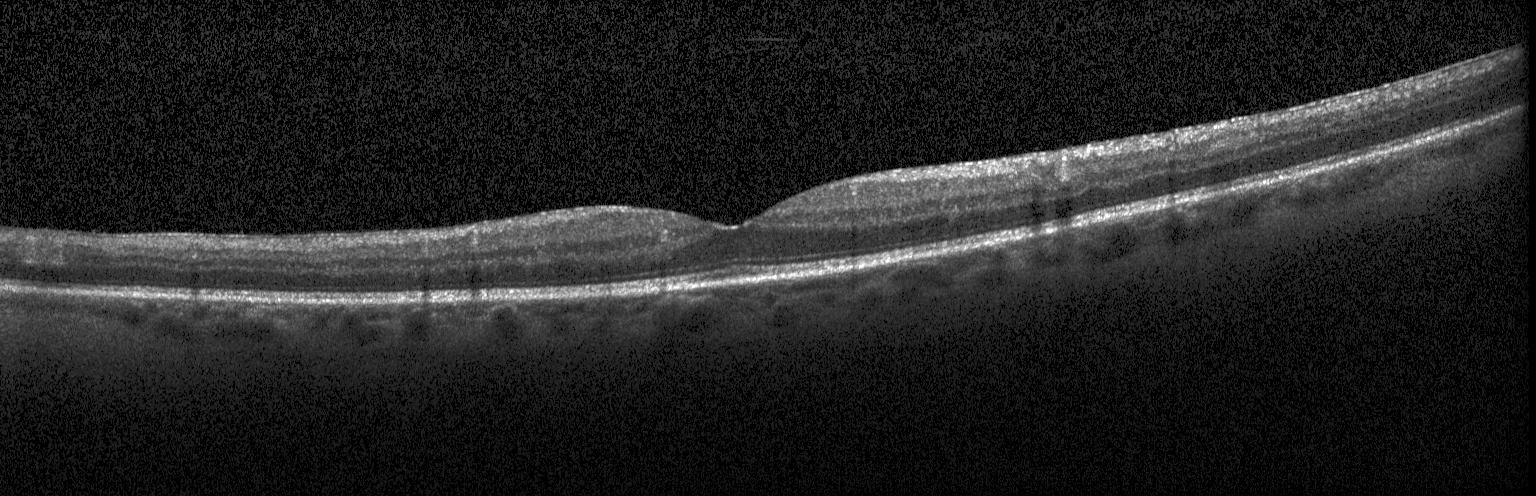

Macular OCT demonstrating no choroidal neovascularization, diabetic macular edema, or drusen.